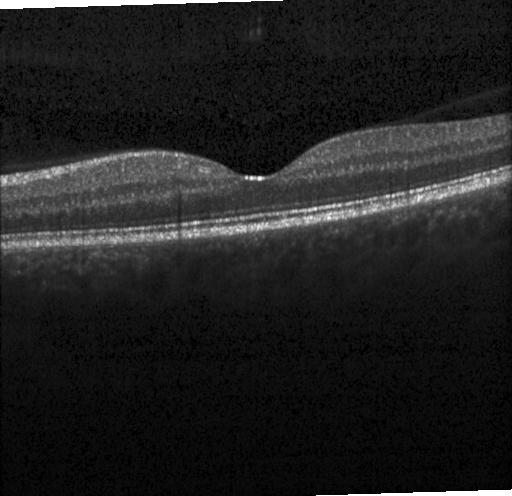 Spectral-domain optical coherence tomography. Acquired on a Heidelberg Spectralis. Optical coherence tomography scan
Diagnosis: no evidence of choroidal neovascularization, diabetic macular edema, or drusen.